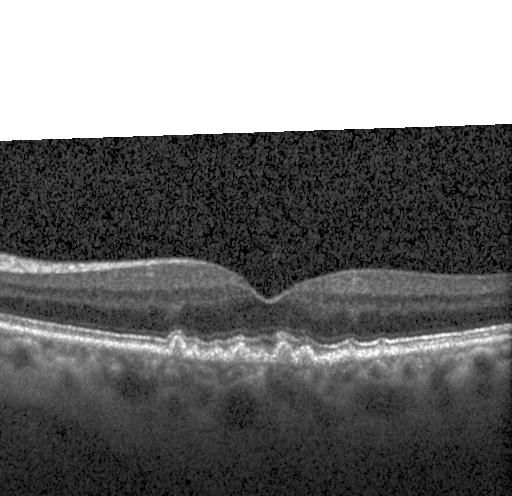 SD-OCT. Heidelberg Spectralis OCT system. OCT line scan — Diagnosis: multiple drusen.